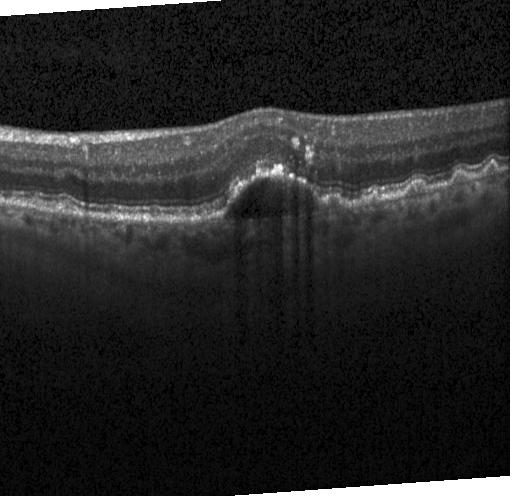 OCT scan showing a choroidal neovascular membrane.